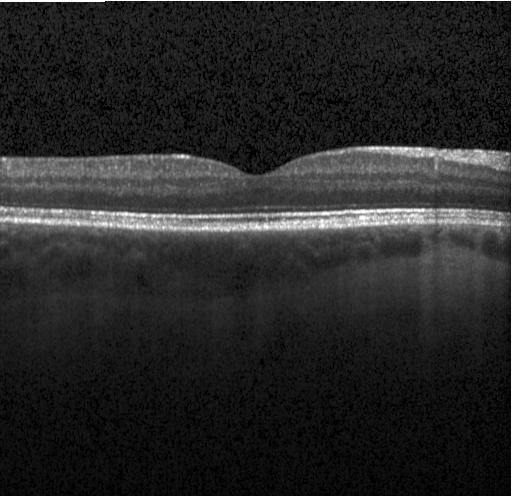
Diagnosis: neither CNV, DME, nor drusen.